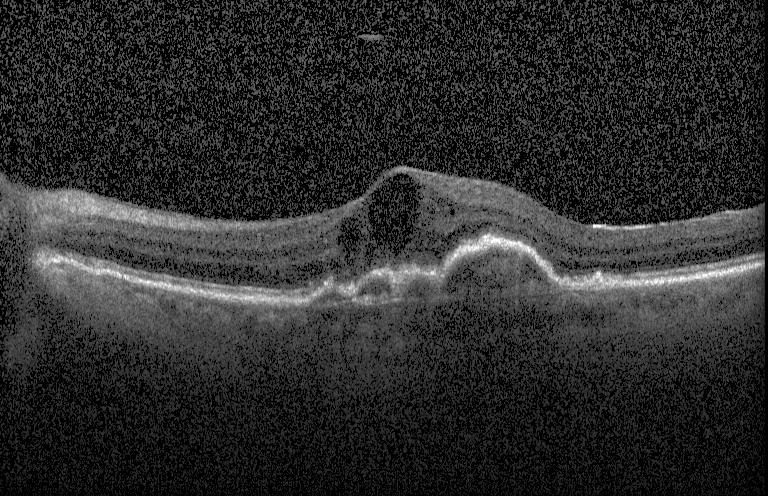

OCT finding: choroidal neovascularization.